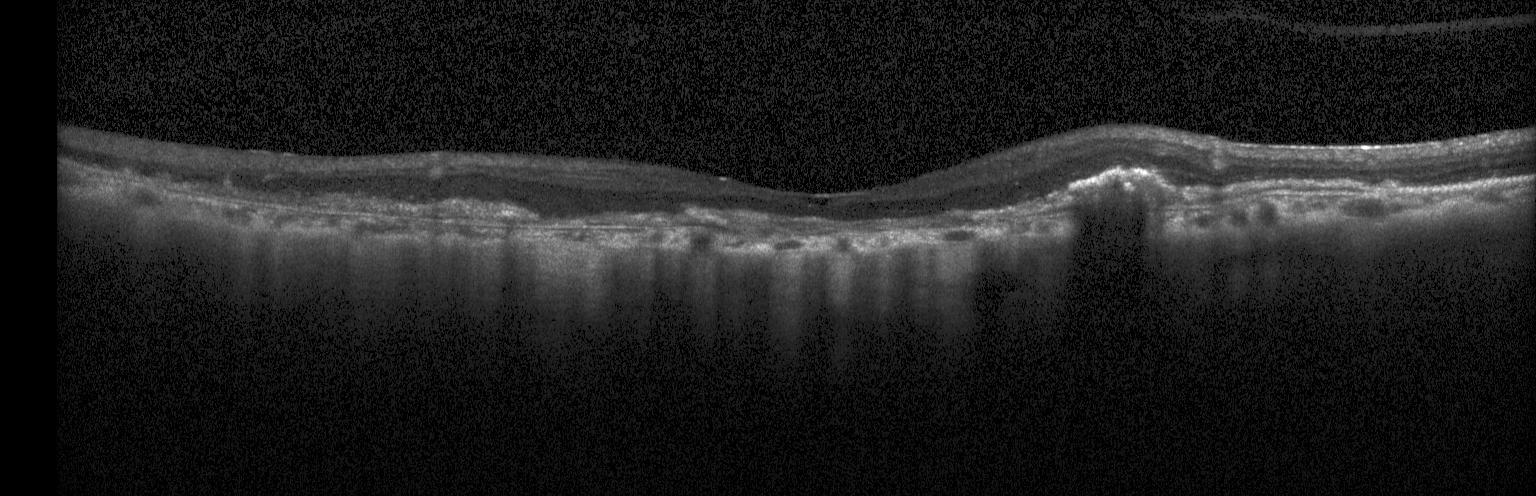
Diagnosis: a choroidal neovascular membrane.